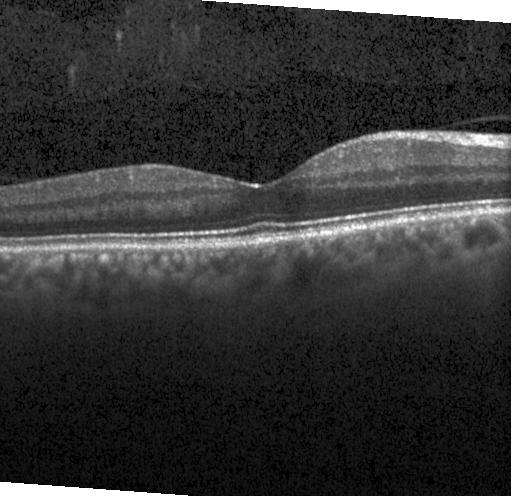
Through the macula; spectral-domain optical coherence tomography; optical coherence tomography B-scan; acquired on a Heidelberg Spectralis.
No evidence of CNV, DME, or drusen.